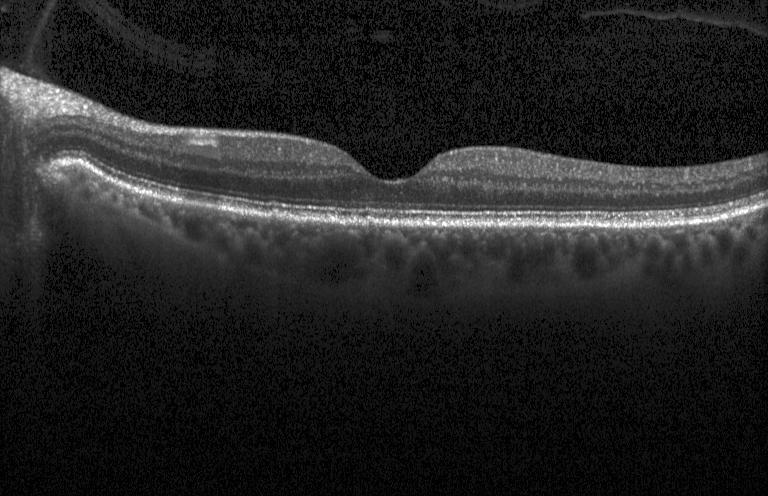

OCT line scan. Assessment: no choroidal neovascularization, diabetic macular edema, or drusen.